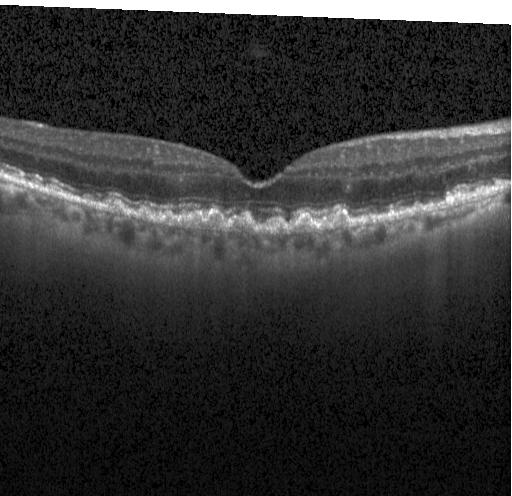

Retinal OCT cross-section.
Impression: multiple drusen.